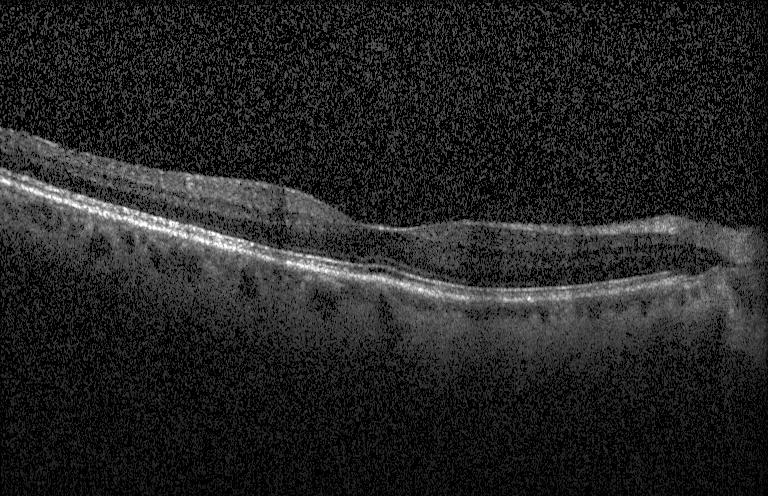
Retinal OCT cross-section. Acquired on a Heidelberg Spectralis. Diagnosis: neither choroidal neovascularization, diabetic macular edema, nor drusen.